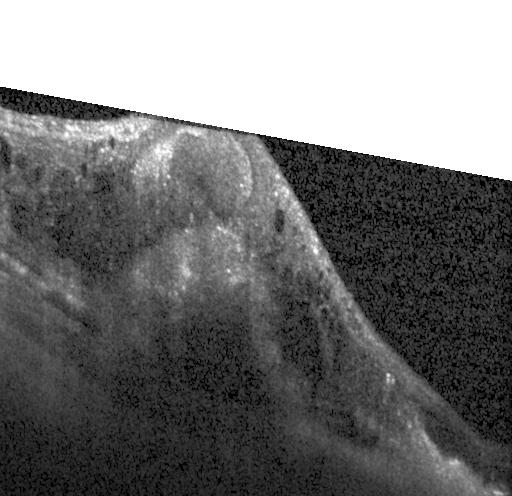

Macular OCT: a choroidal neovascular membrane.